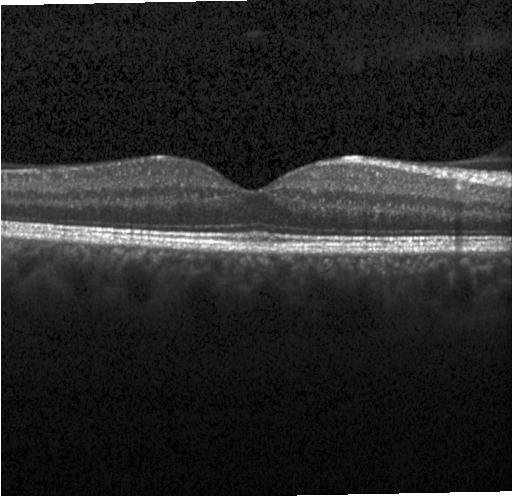
OCT B-scan. OCT finding: no evidence of choroidal neovascularization, diabetic macular edema, or drusen.